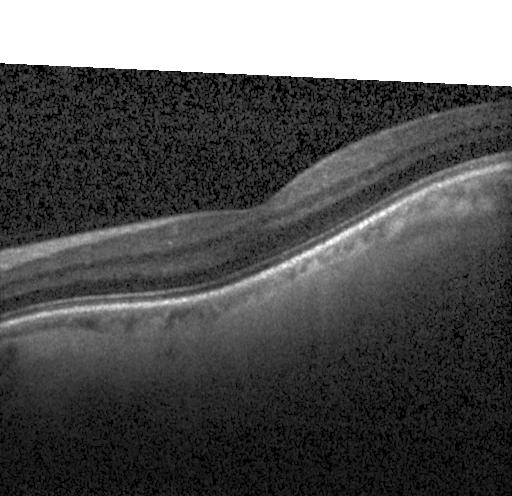

Macular OCT: neither CNV, DME, nor drusen.